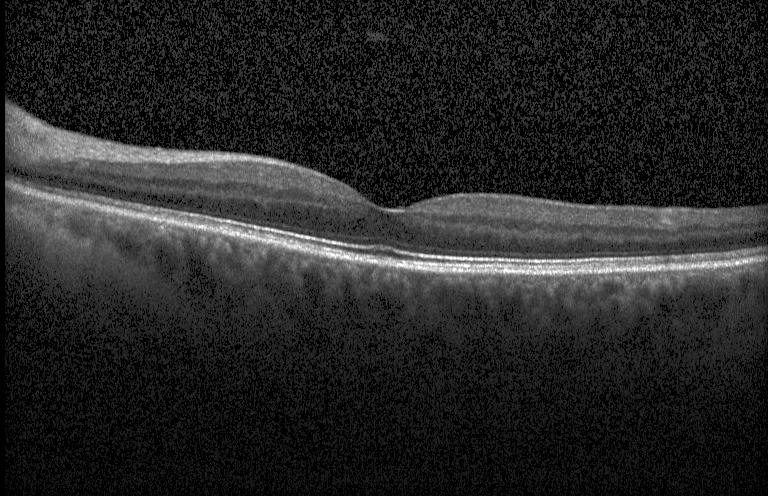 Spectral-domain OCT, acquired on a Heidelberg Spectralis, OCT line scan.
Finding: no choroidal neovascularization, no diabetic macular edema, and no drusen.